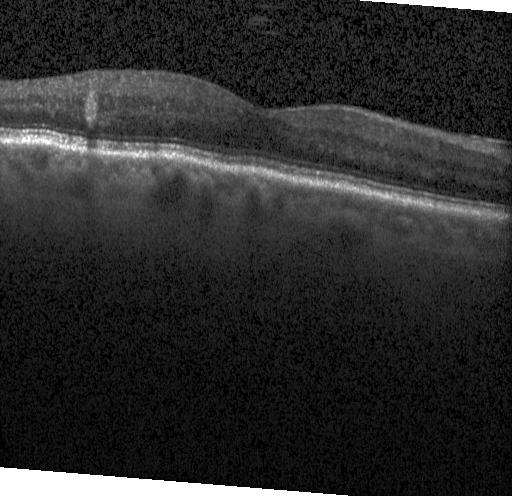 Optical coherence tomography scan; spectral-domain OCT — No CNV, no DME, and no drusen.